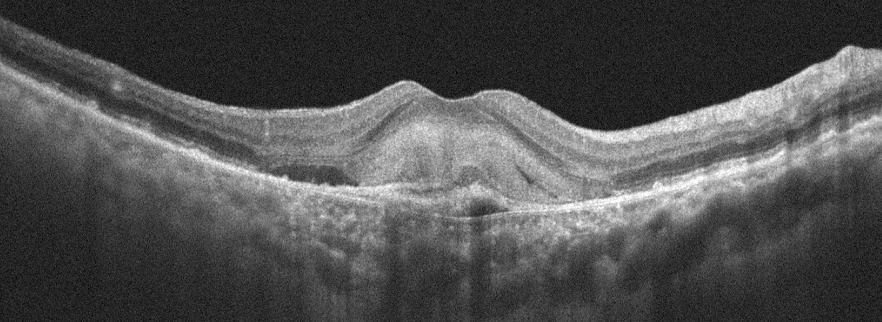

Oculus sinister; optical coherence tomography B-scan. Macular OCT: age-related macular degeneration.